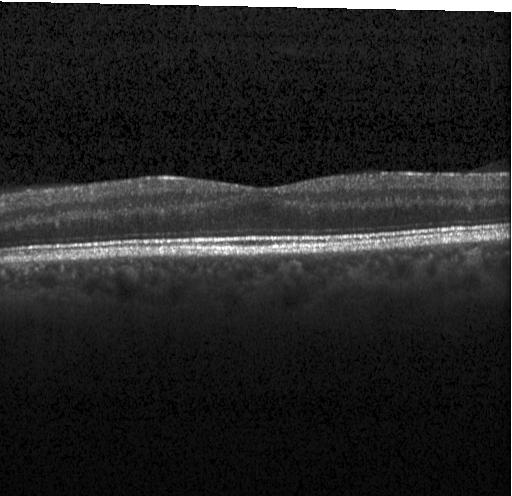
Horizontal scan through the fovea, optical coherence tomography scan. This B-scan demonstrates neither choroidal neovascularization, diabetic macular edema, nor drusen.